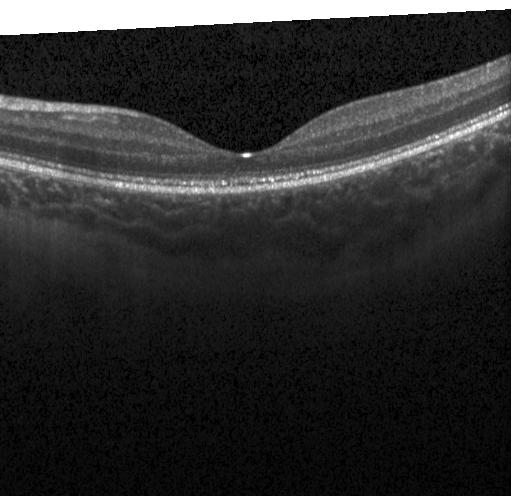

Macular OCT: neither choroidal neovascularization, diabetic macular edema, nor drusen.